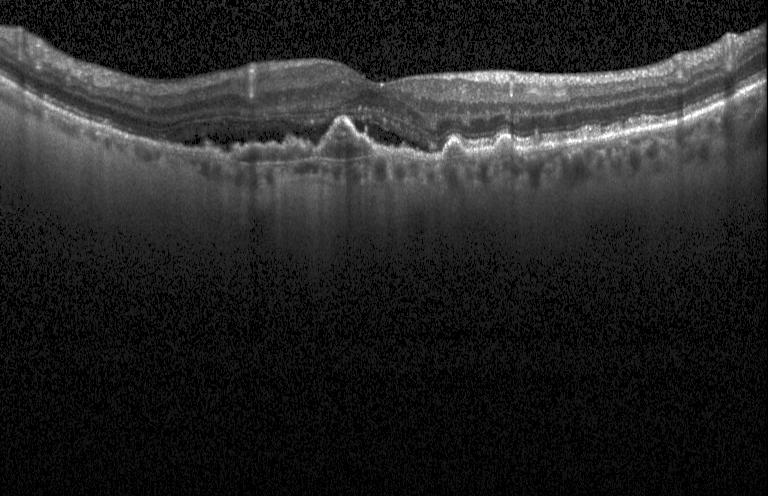 SD-OCT. Heidelberg Spectralis OCT system. Fovea-centered. Optical coherence tomography B-scan.
Macular OCT: a choroidal neovascular membrane.